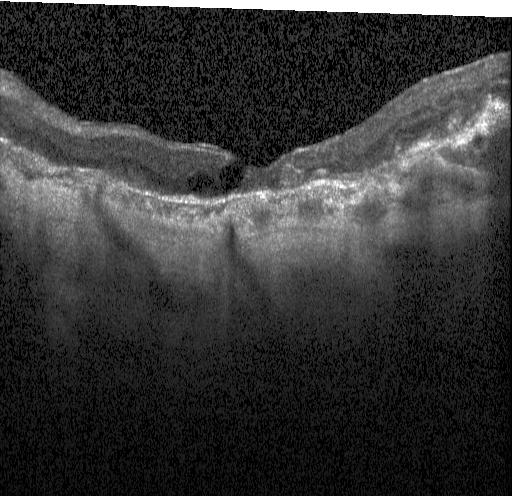 Retinal OCT cross-section showing a choroidal neovascular membrane.